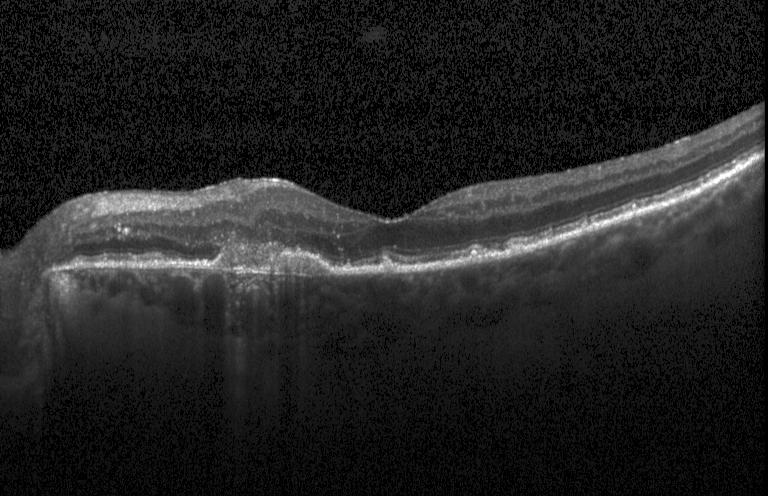
Heidelberg Spectralis, optical coherence tomography B-scan, macular scan, spectral-domain OCT.
Diagnosis: CNV.